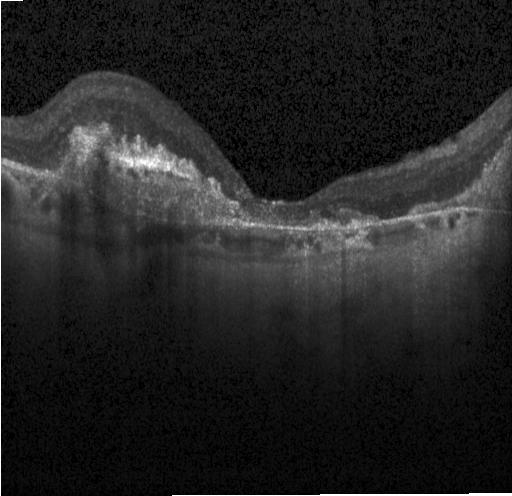
Instrument: Heidelberg Spectralis, fovea-centered, retinal OCT cross-section, spectral-domain OCT. Impression: CNV.